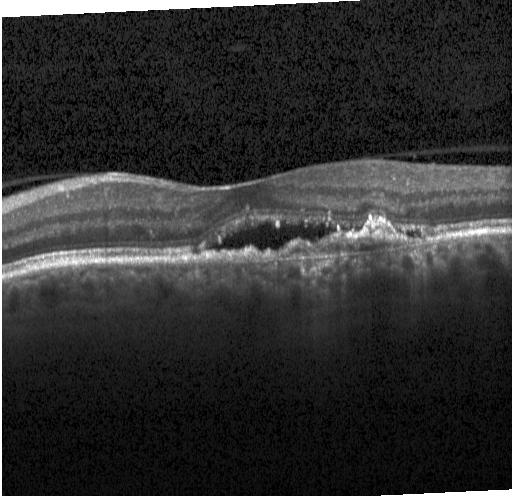
Retinal OCT B-scan, centered on the fovea.
Impression: a choroidal neovascular membrane.